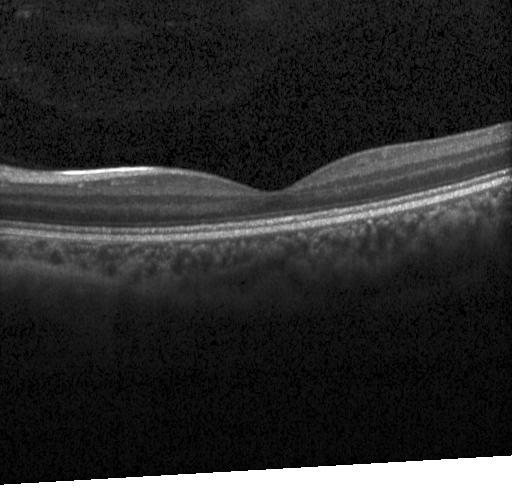
Acquired on a Heidelberg Spectralis; optical coherence tomography B-scan. Impression: neither choroidal neovascularization, diabetic macular edema, nor drusen.